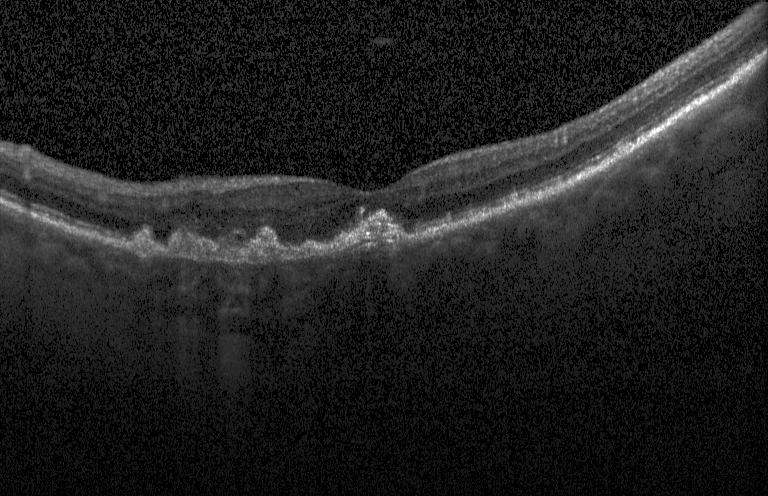

Spectral-domain optical coherence tomography; retinal OCT B-scan — Dx: choroidal neovascularization (CNV).